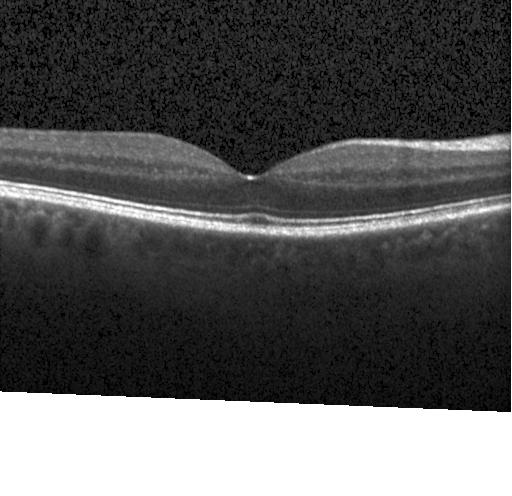
Diagnosis: neither CNV, DME, nor drusen.